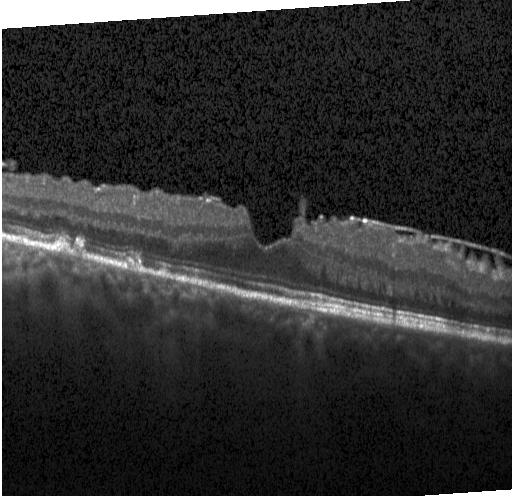 Spectral-domain OCT B-scan: drusen.